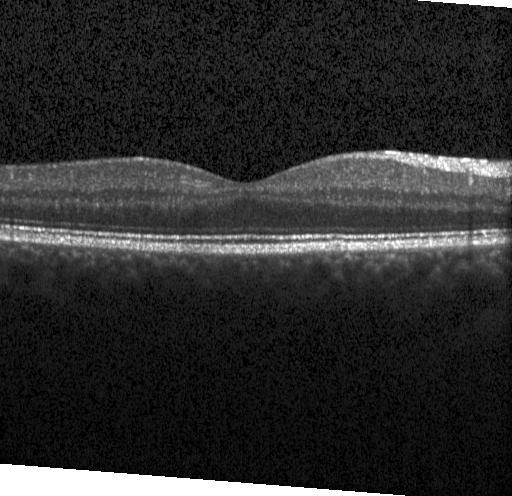

Impression: no evidence of CNV, DME, or drusen.